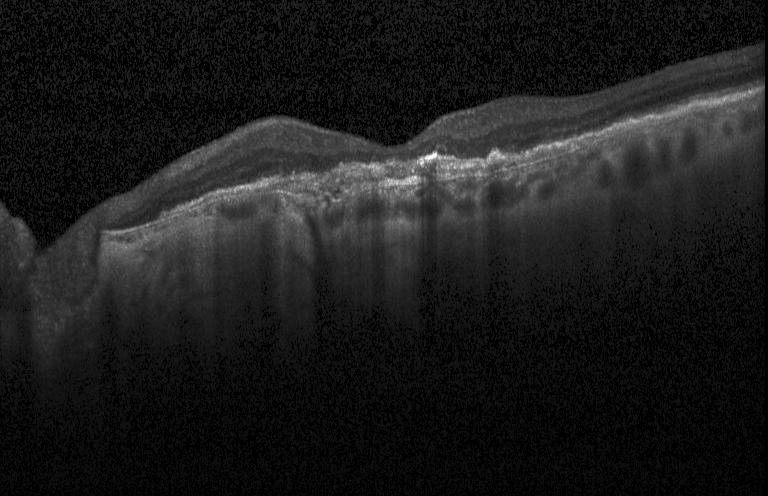

Centered on the fovea, spectral-domain optical coherence tomography, acquired on a Heidelberg Spectralis, optical coherence tomography scan.
Diagnosis: choroidal neovascularization.